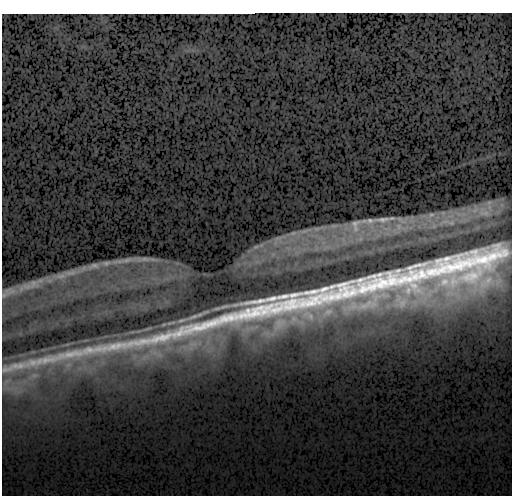
Retinal OCT B-scan; spectral-domain optical coherence tomography
Dx: neither choroidal neovascularization, diabetic macular edema, nor drusen.